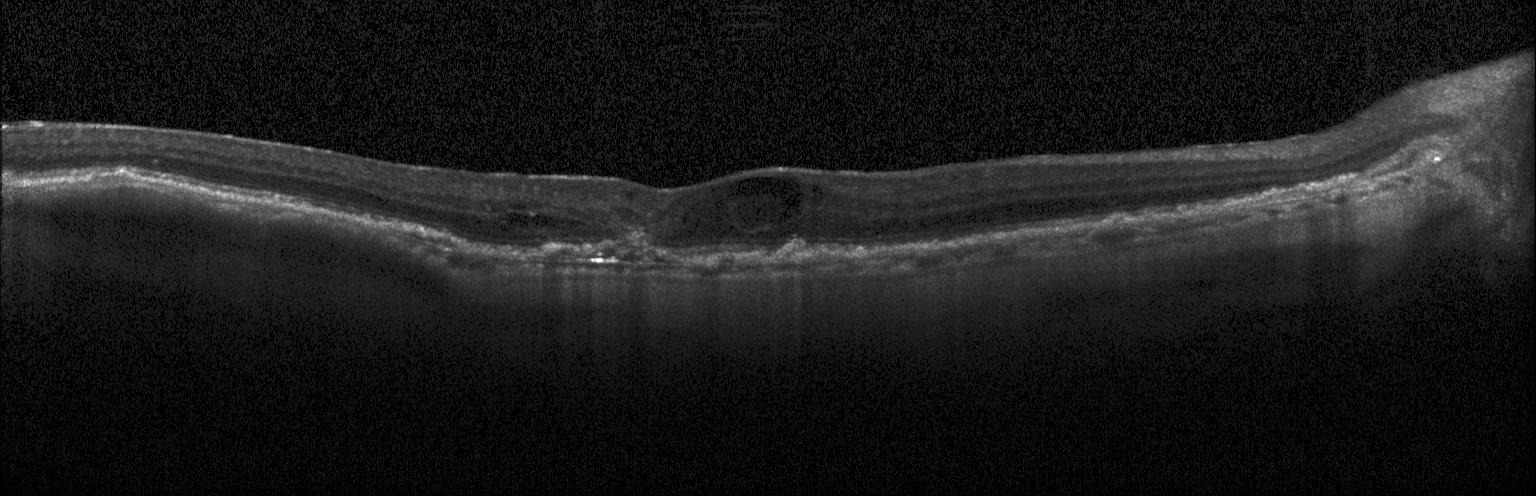

Retinal OCT cross-section showing choroidal neovascularization (CNV).